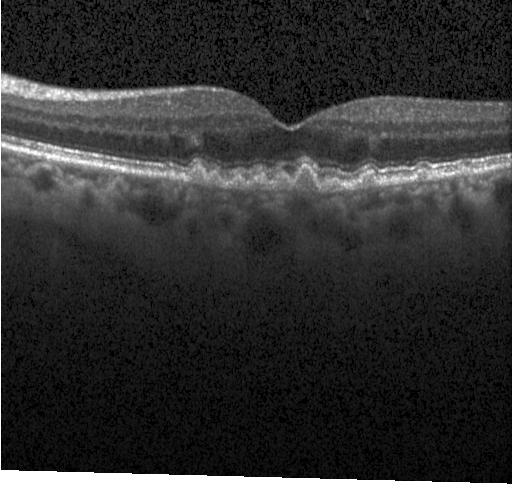 OCT B-scan — Dx: drusen.